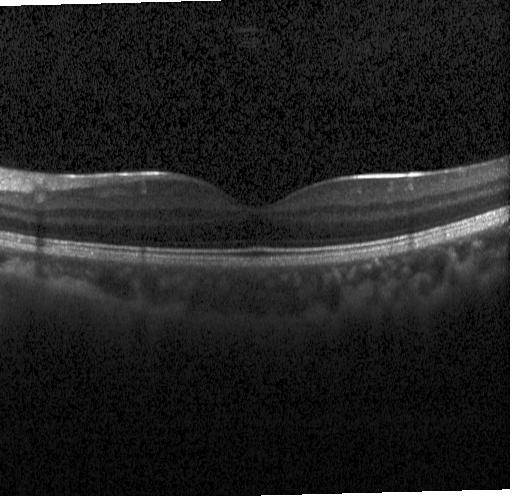 Acquired on a Heidelberg Spectralis. Optical coherence tomography B-scan
The scan shows no evidence of CNV, DME, or drusen.